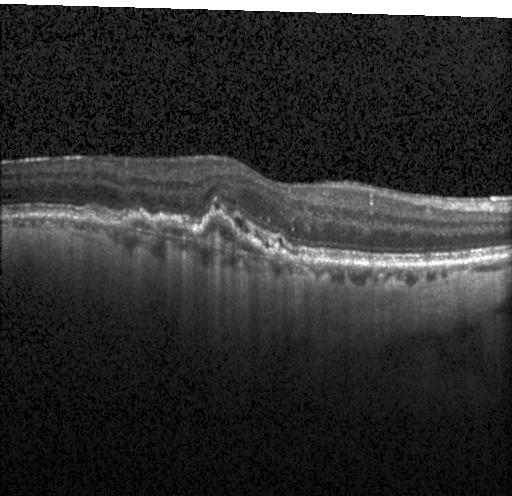 OCT B-scan, fovea-centered, SD-OCT, Heidelberg Spectralis OCT system — This B-scan demonstrates choroidal neovascularization (CNV).